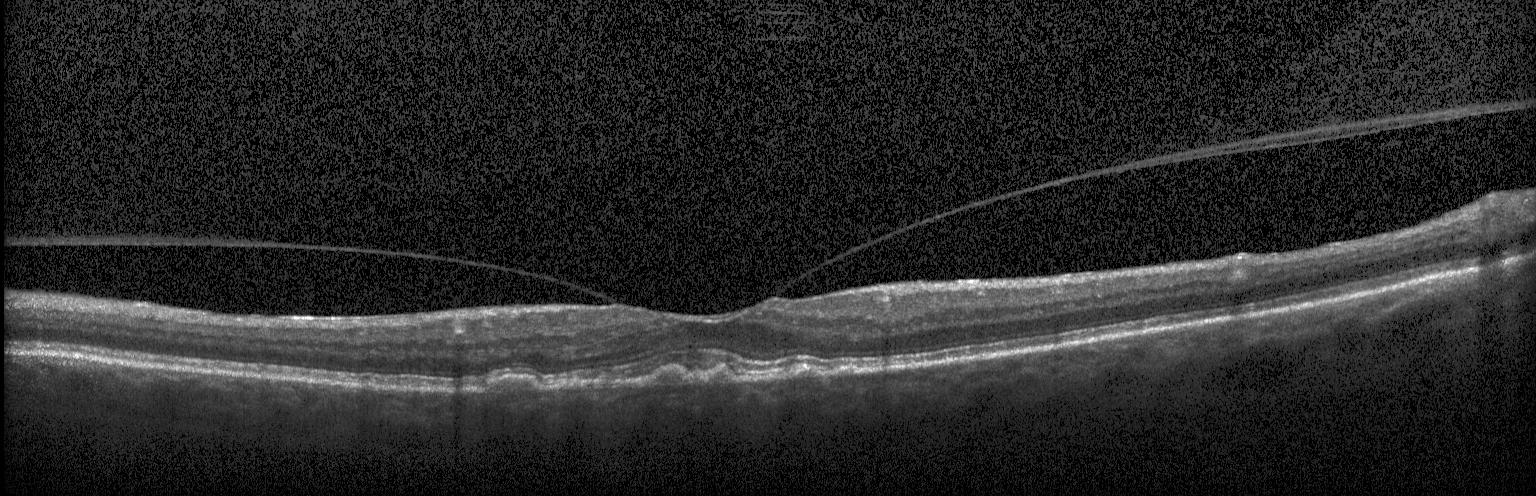
Dx: sub-RPE drusenoid deposits.